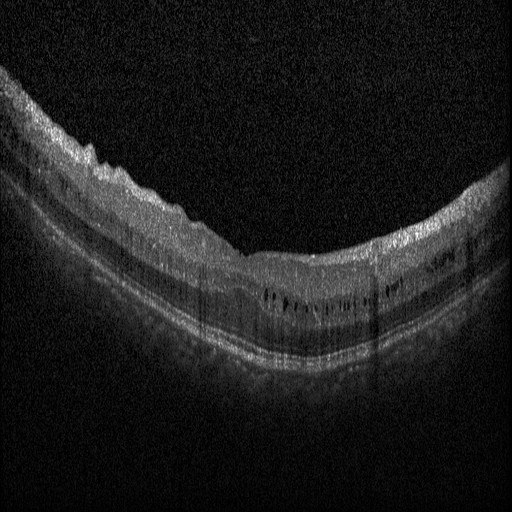 Optical coherence tomography scan, instrument: Heidelberg Spectralis
DME.